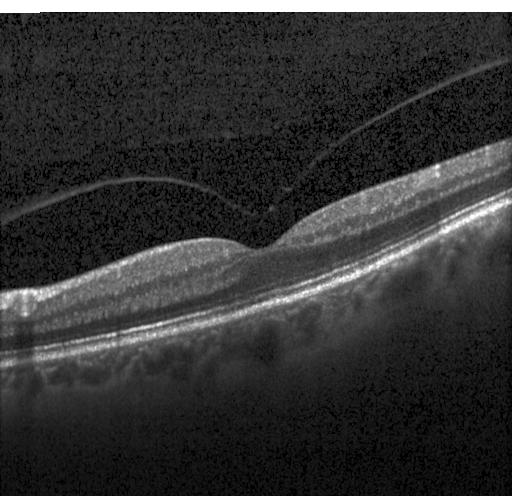 Retinal OCT B-scan.
Impression: no CNV, DME, or drusen.